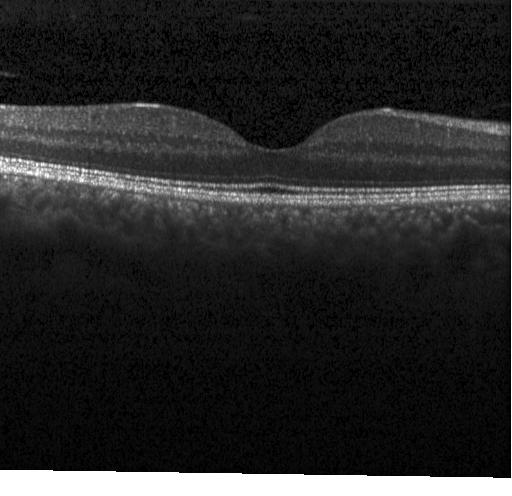
Optical coherence tomography B-scan · spectral-domain optical coherence tomography · fovea-centered. Diagnosis: no evidence of choroidal neovascularization, diabetic macular edema, or drusen.